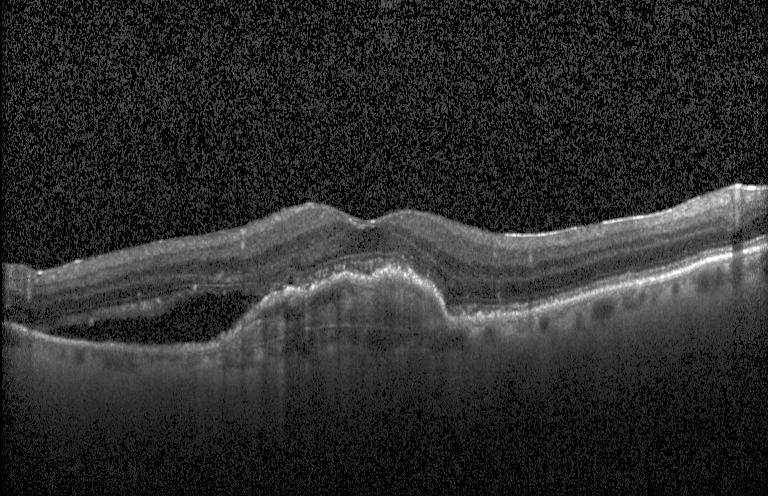 Diagnosis: a choroidal neovascular membrane.